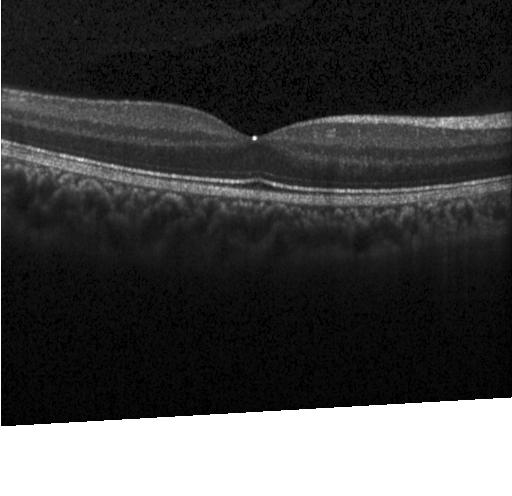 Dx: no CNV, no DME, and no drusen.